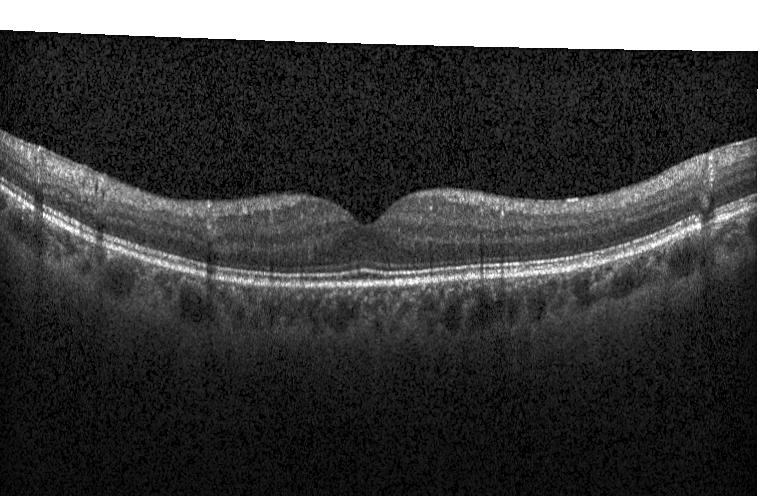 Through the macula. Retinal OCT cross-section. Spectral-domain optical coherence tomography. Macular OCT: no CNV, no DME, and no drusen.